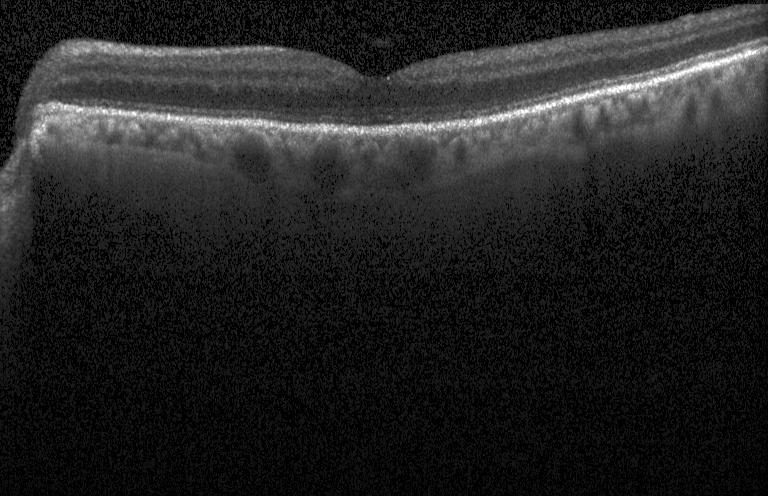
Heidelberg Spectralis. Retinal OCT B-scan. Macular scan. Spectral-domain OCT. Finding: no CNV, DME, or drusen.